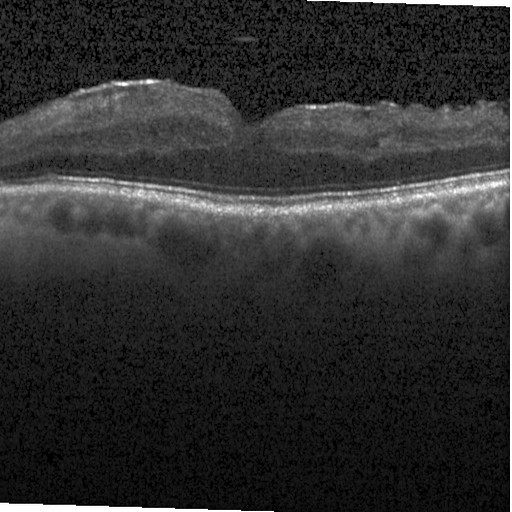
OCT line scan; spectral-domain optical coherence tomography — Diabetic macular edema (DME).